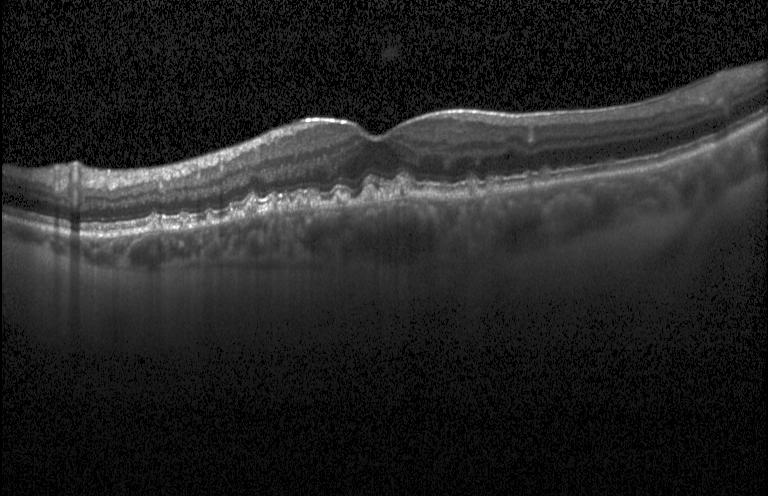

Diagnosis: multiple drusen.